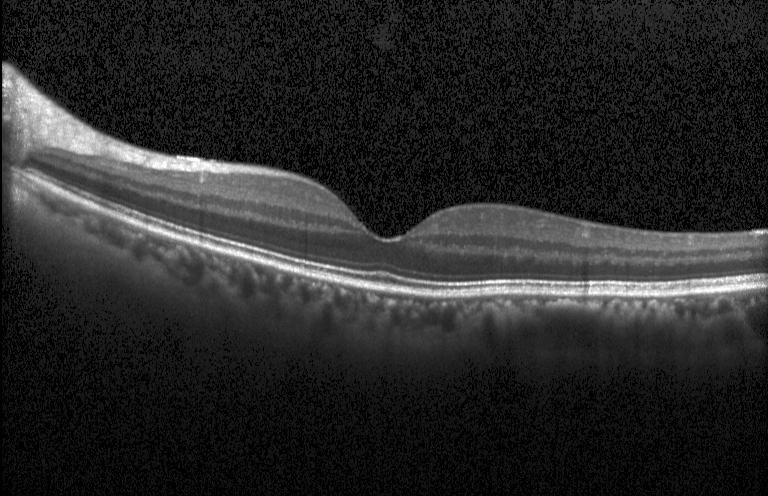 OCT line scan. Diagnosis: neither choroidal neovascularization, diabetic macular edema, nor drusen.